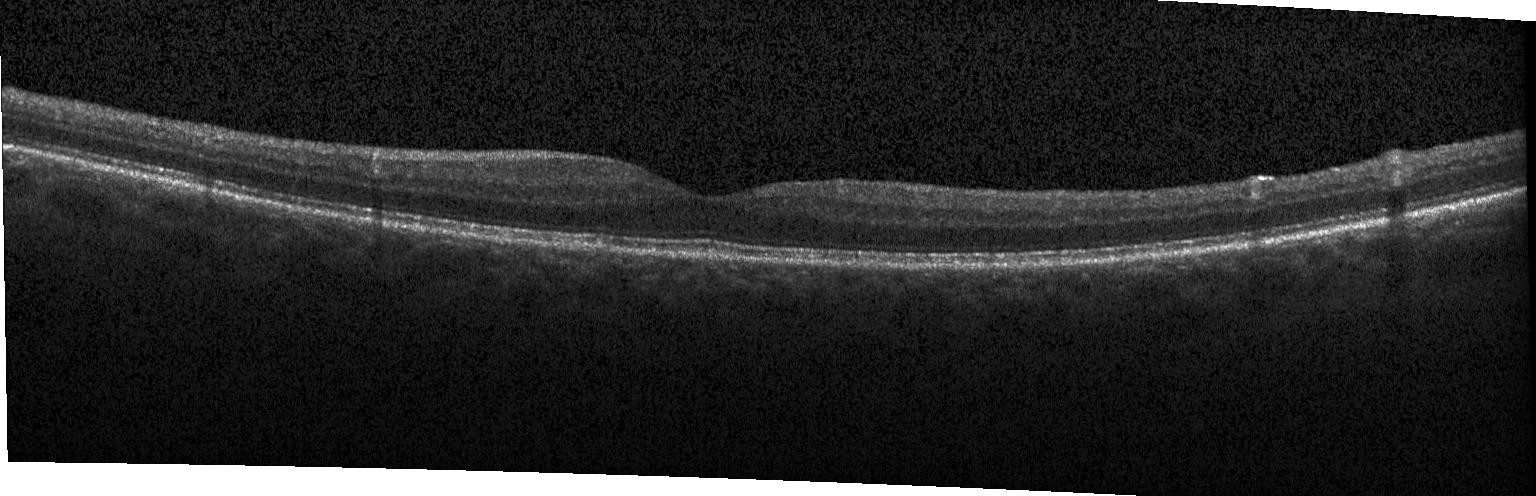 Centered on the fovea. Spectral-domain OCT. Acquired on a Heidelberg Spectralis. OCT line scan
Finding: no CNV, DME, or drusen.